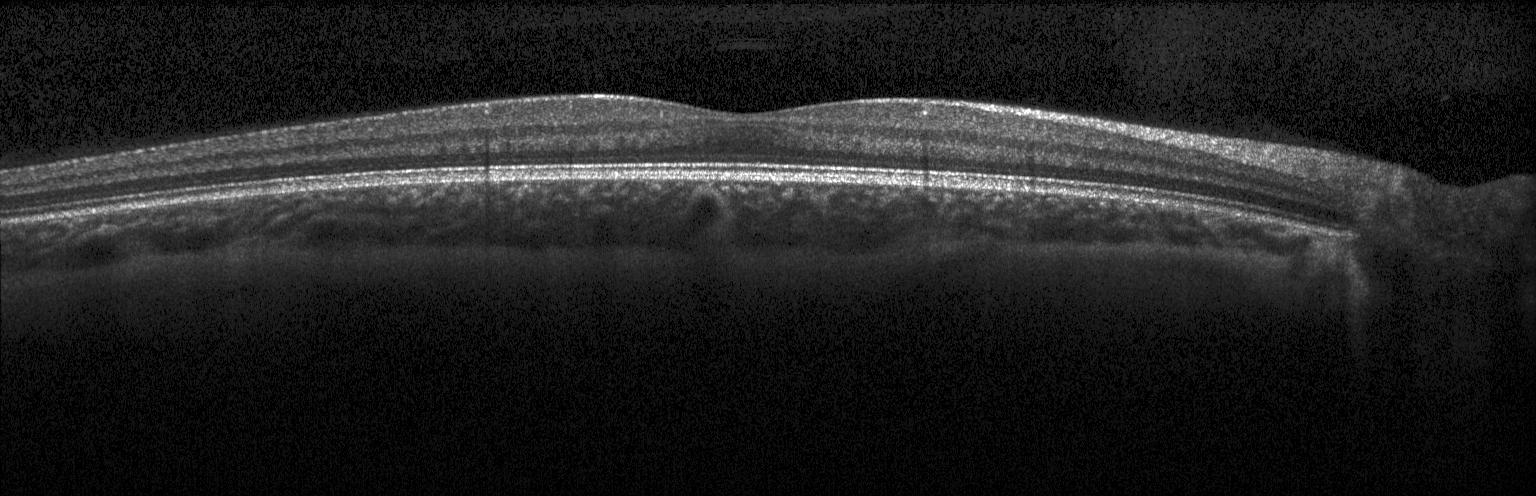 Through the macula. Retinal OCT cross-section. SD-OCT.
Finding: neither CNV, DME, nor drusen.